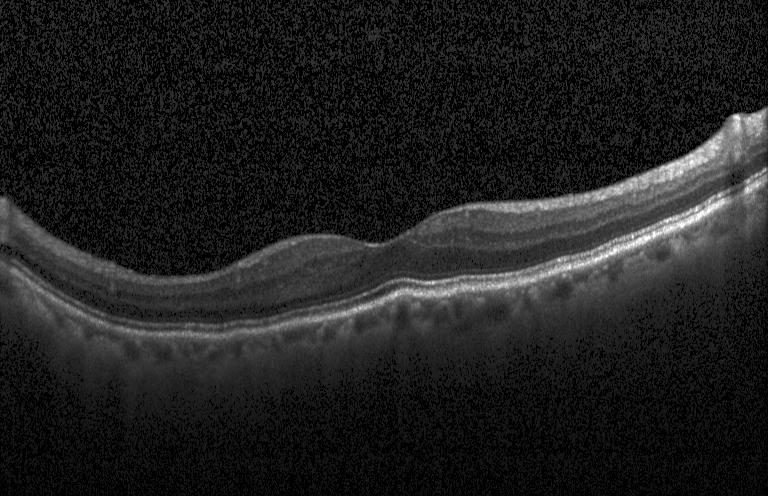

Acquired on a Heidelberg Spectralis. OCT B-scan
Dx: no choroidal neovascularization, no diabetic macular edema, and no drusen.